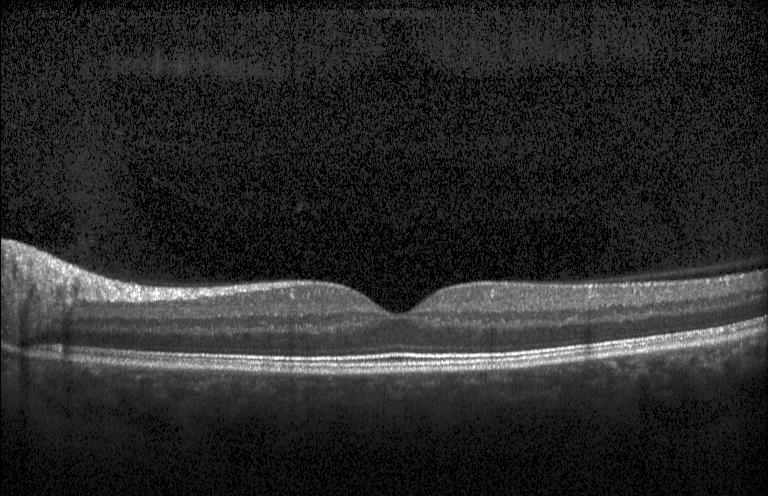 Impression: no CNV, DME, or drusen.